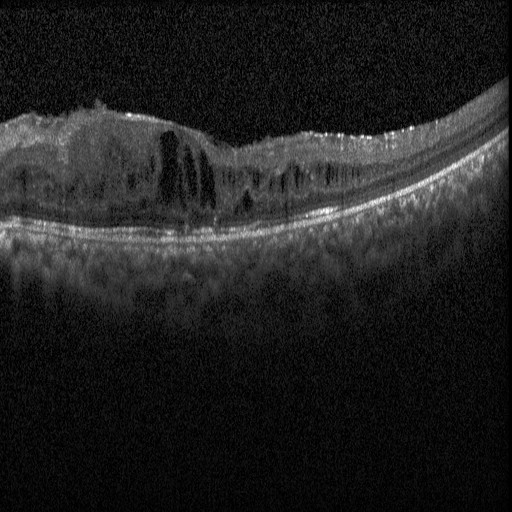

Optical coherence tomography scan, centered on the fovea, Heidelberg Spectralis OCT system, SD-OCT. Macular OCT: DME.